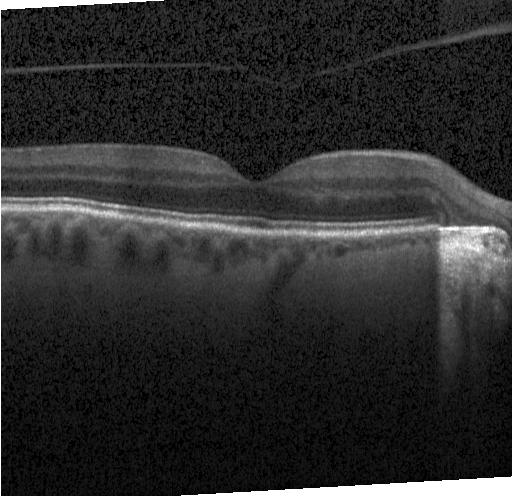 Retinal OCT cross-section · Heidelberg Spectralis · centered on the fovea. This B-scan demonstrates no evidence of choroidal neovascularization, diabetic macular edema, or drusen.